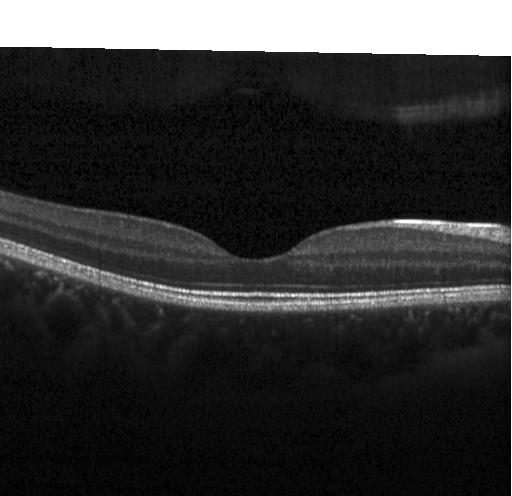 Diagnosis: neither choroidal neovascularization, diabetic macular edema, nor drusen.